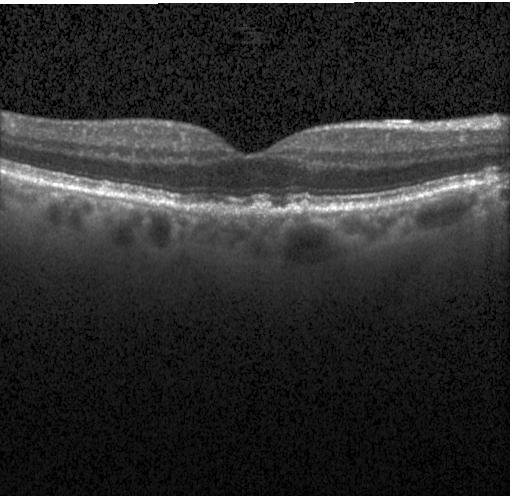 Acquired on a Heidelberg Spectralis, spectral-domain optical coherence tomography, retinal OCT cross-section, centered on the fovea. Diagnosis: sub-RPE drusenoid deposits.